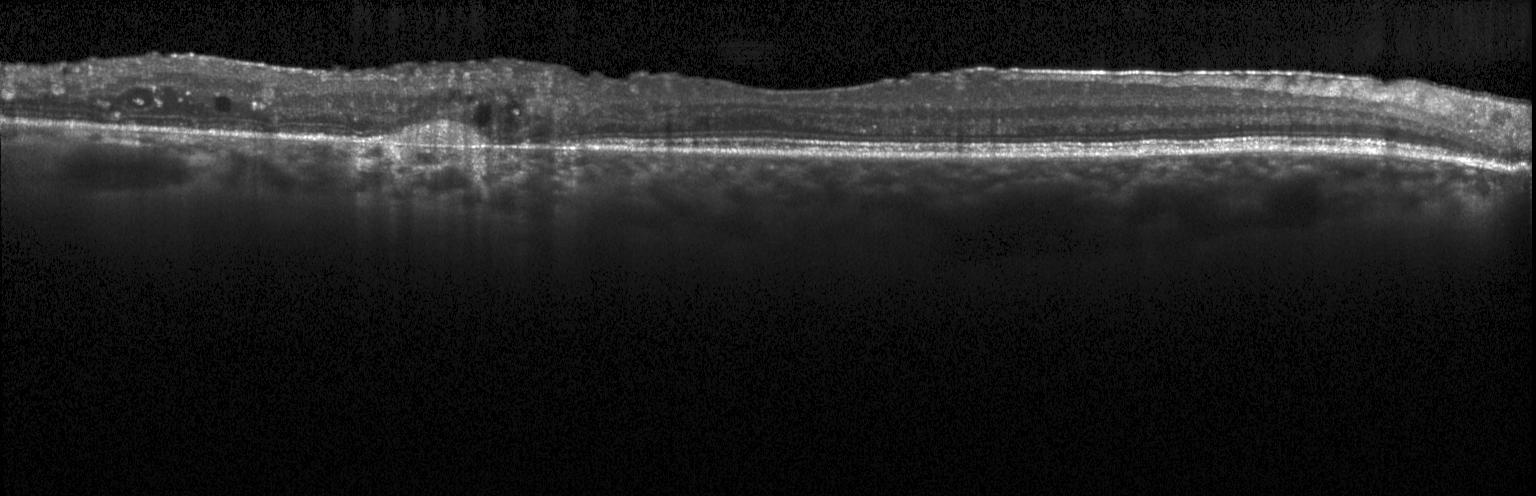
Heidelberg Spectralis · macular scan · spectral-domain OCT · OCT line scan.
CNV.